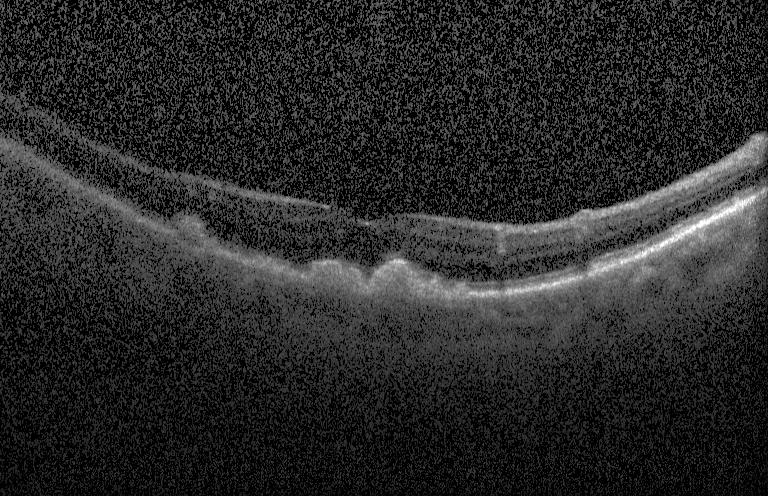

Macular OCT: drusen.